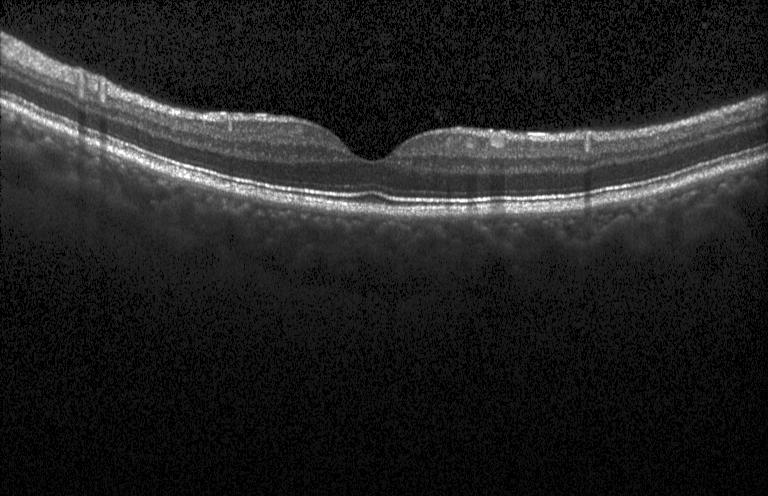

Spectral-domain OCT · Heidelberg Spectralis OCT system · retinal OCT B-scan.
The scan shows no evidence of CNV, DME, or drusen.